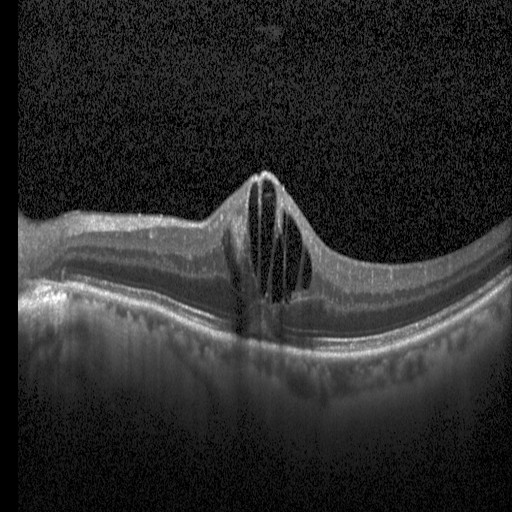 Assessment: diabetic macular edema.